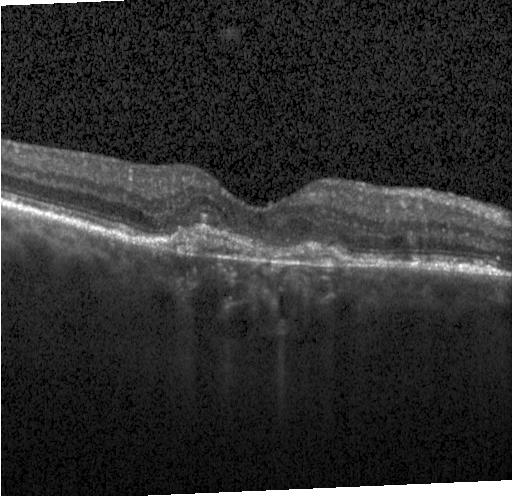

Diagnosis: choroidal neovascularization (CNV).